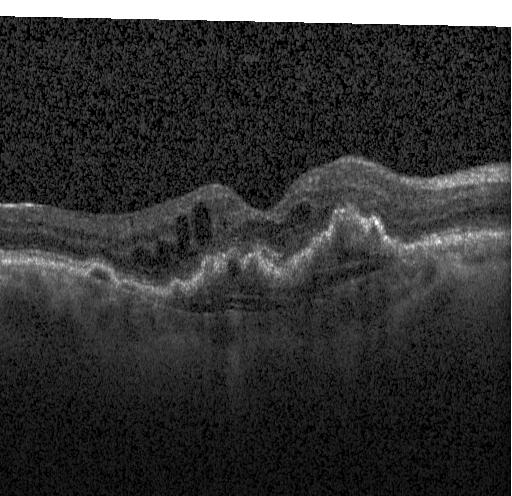 Spectral-domain OCT B-scan: choroidal neovascularization (CNV).